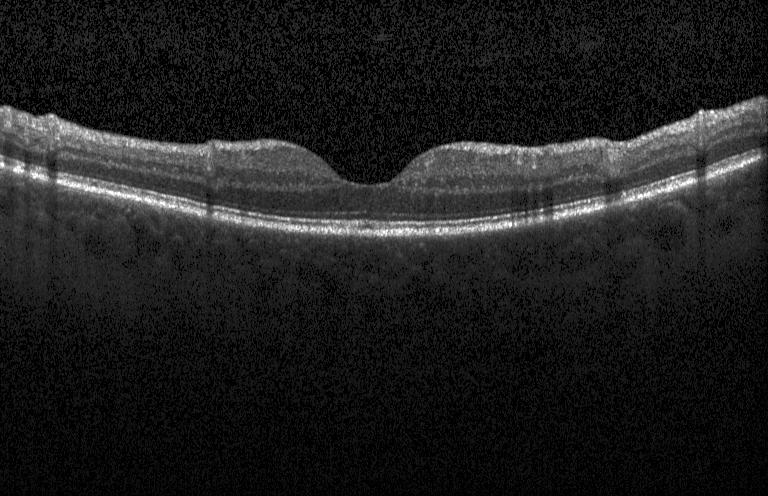 Finding: no evidence of choroidal neovascularization, diabetic macular edema, or drusen.